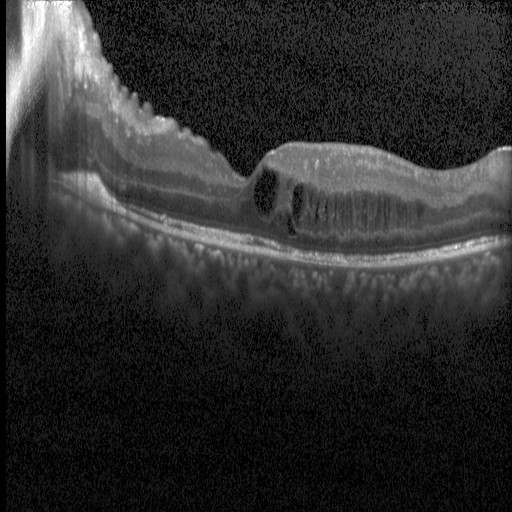 Diagnosis: DME.